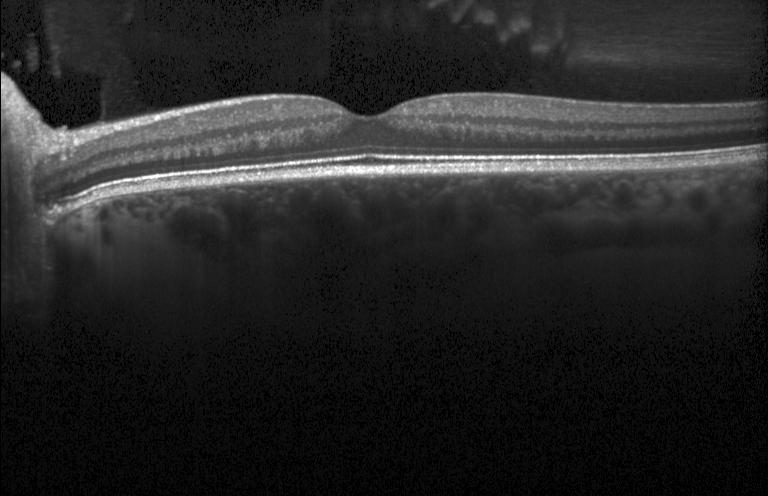 Retinal OCT B-scan. Fovea-centered. Instrument: Heidelberg Spectralis — Assessment: no choroidal neovascularization, no diabetic macular edema, and no drusen.